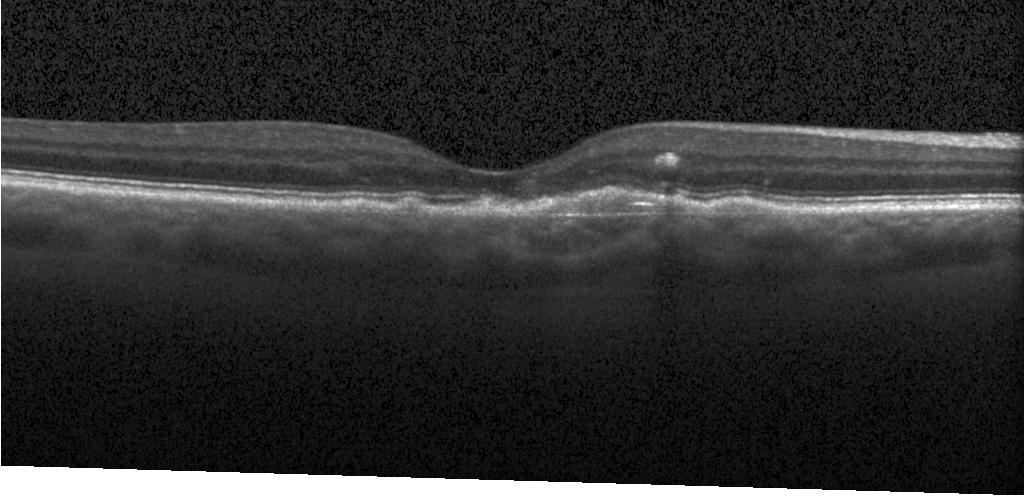 Instrument: Heidelberg Spectralis, optical coherence tomography scan — This B-scan demonstrates a choroidal neovascular membrane.